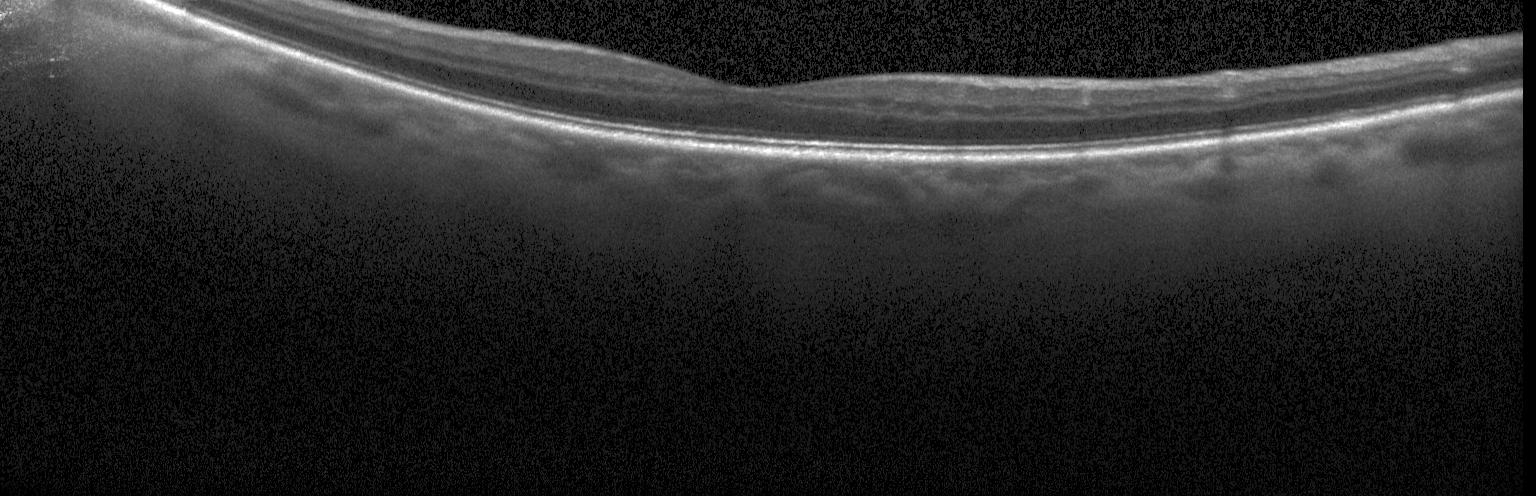

Heidelberg Spectralis; spectral-domain optical coherence tomography; optical coherence tomography scan; fovea-centered — Diagnosis: no choroidal neovascularization, diabetic macular edema, or drusen.